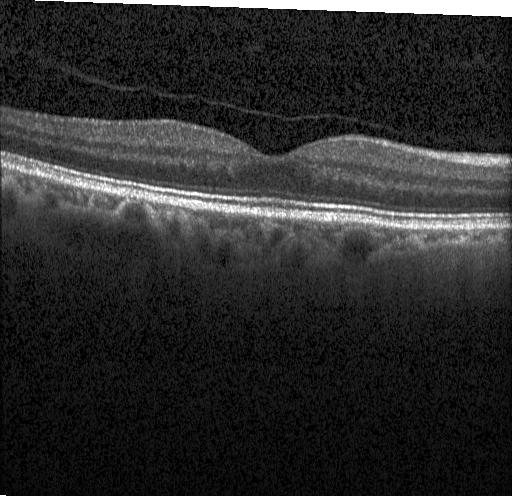

OCT B-scan showing neither choroidal neovascularization, diabetic macular edema, nor drusen.